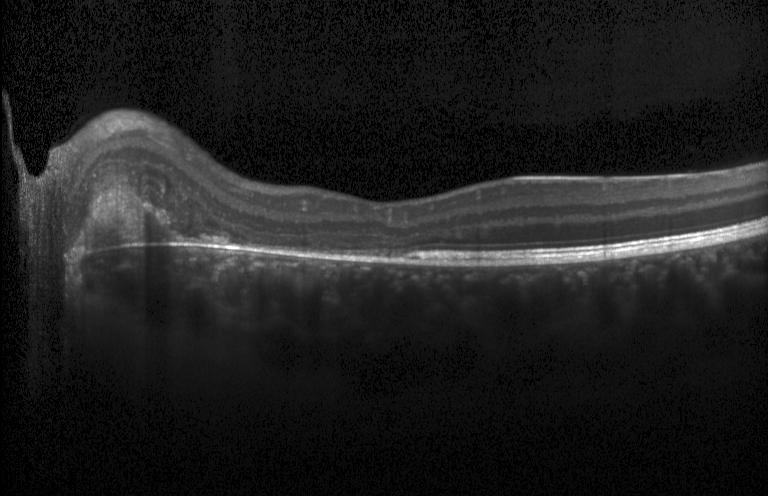
A choroidal neovascular membrane.